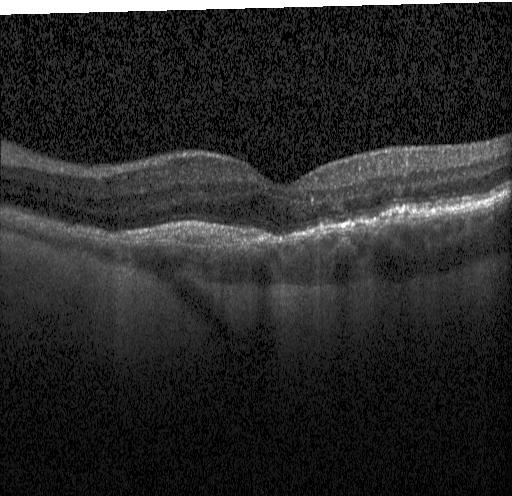 OCT B-scan. Finding: a choroidal neovascular membrane.